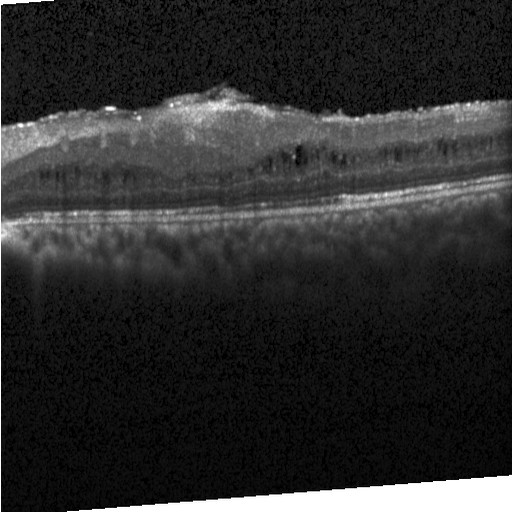 OCT line scan.
Assessment: diabetic macular edema (DME).